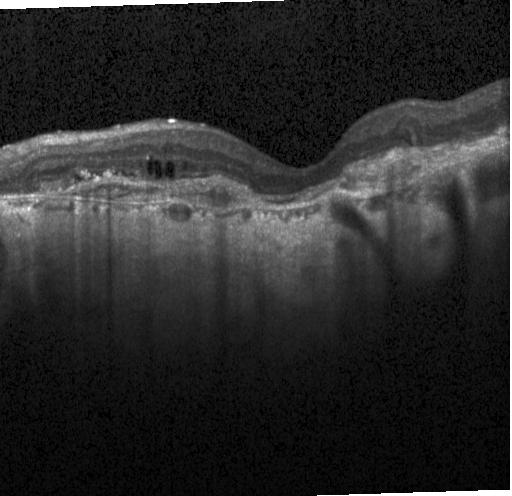

Acquired on a Heidelberg Spectralis; spectral-domain OCT; optical coherence tomography B-scan
Dx: a choroidal neovascular membrane.